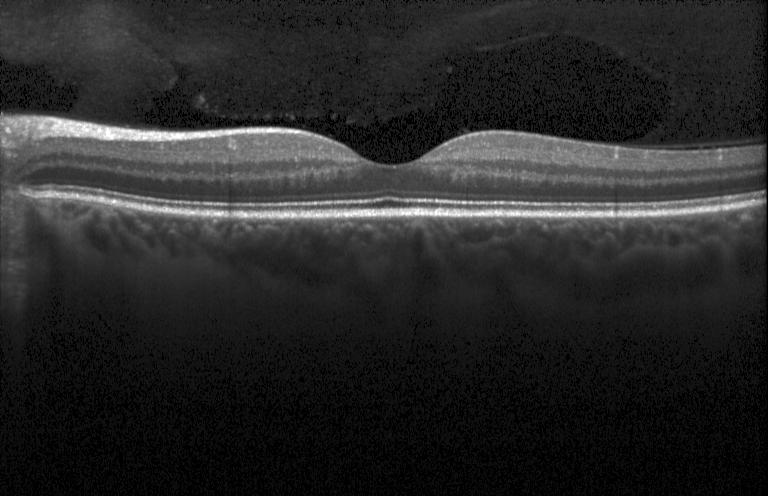 Spectral-domain OCT. Optical coherence tomography B-scan. Horizontal scan through the fovea. Acquired on a Heidelberg Spectralis.
The scan shows no choroidal neovascularization, diabetic macular edema, or drusen.